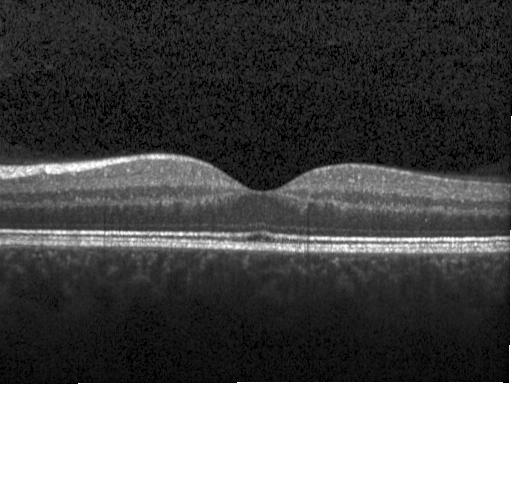
Assessment: neither CNV, DME, nor drusen.